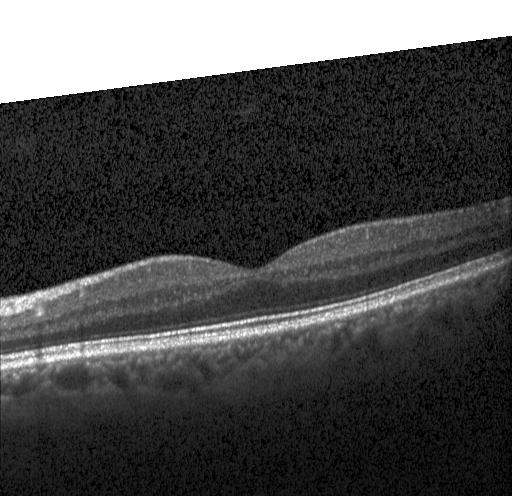

Fovea-centered, retinal OCT B-scan
Impression: no CNV, DME, or drusen.